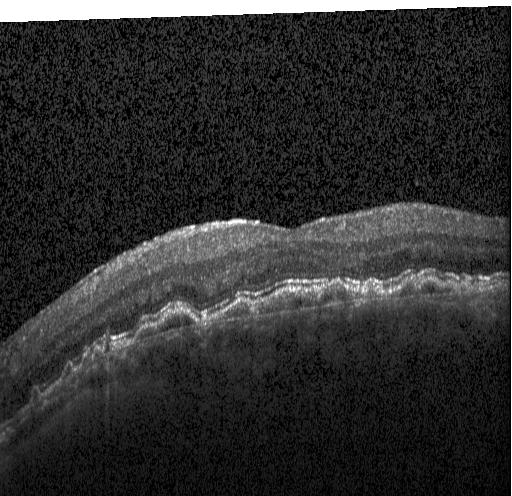

Horizontal scan through the fovea, acquired on a Heidelberg Spectralis, optical coherence tomography B-scan, spectral-domain OCT
Impression: choroidal neovascularization.